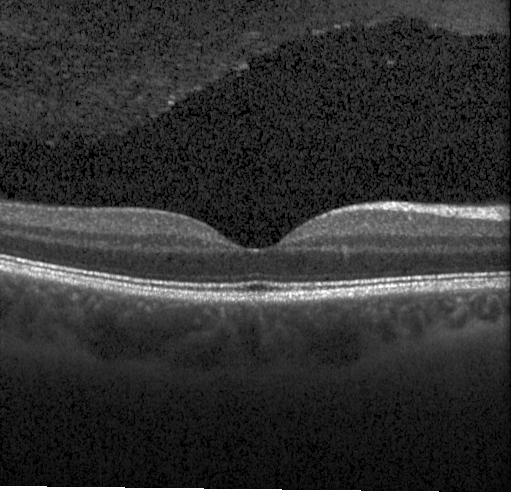 OCT B-scan.
Dx: no choroidal neovascularization, no diabetic macular edema, and no drusen.